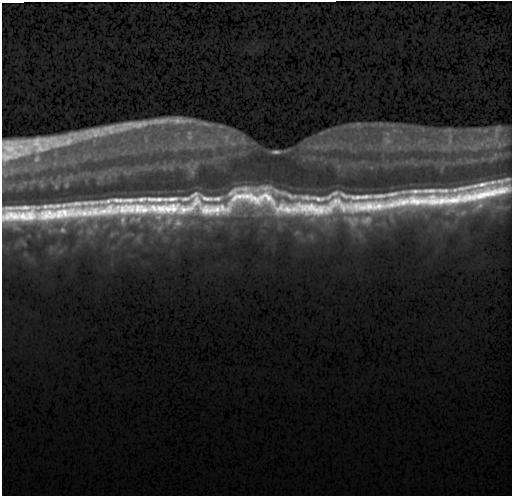
Diagnosis: multiple drusen.